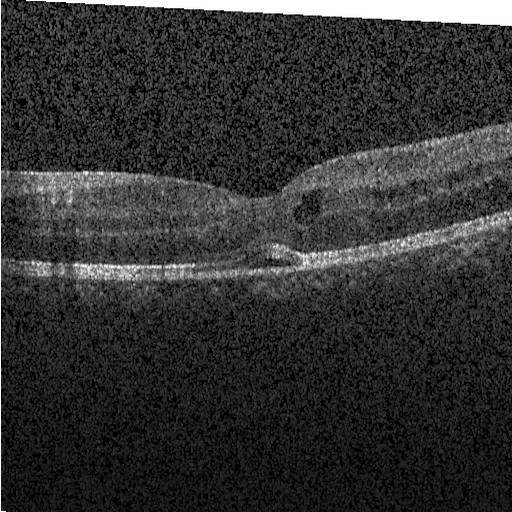
Optical coherence tomography B-scan · spectral-domain optical coherence tomography · Heidelberg Spectralis · centered on the fovea
Diagnosis: DME.